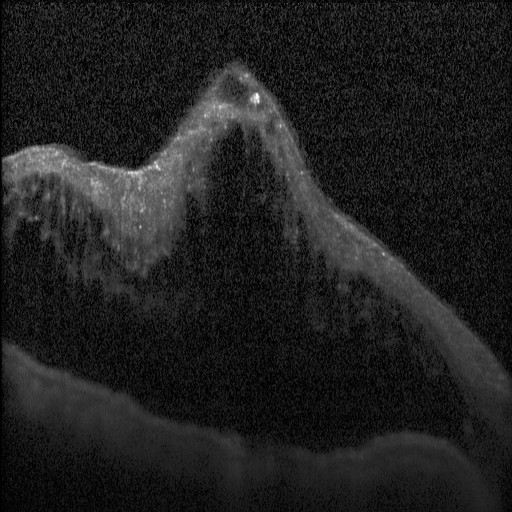 Optical coherence tomography scan. Heidelberg Spectralis. Spectral-domain optical coherence tomography — Impression: DME.